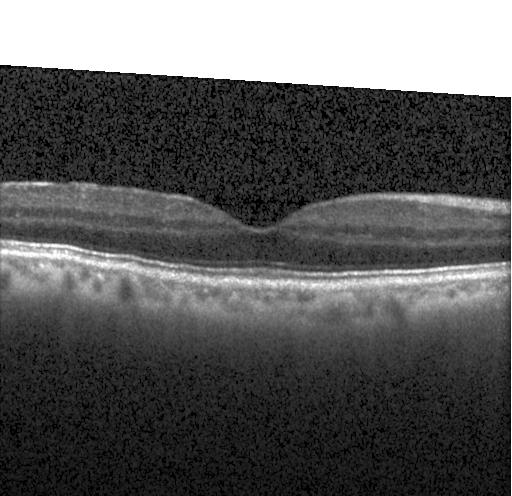
This B-scan demonstrates neither CNV, DME, nor drusen.